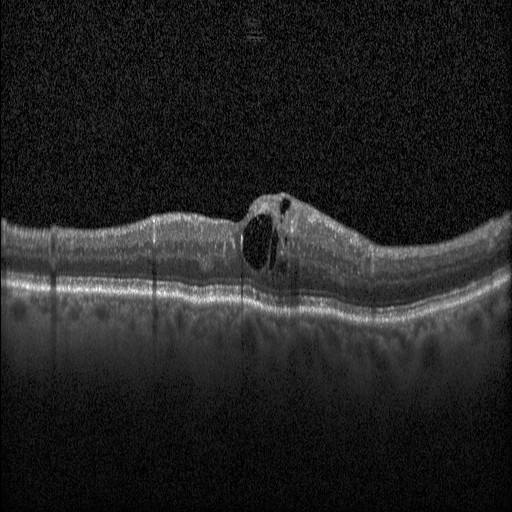
SD-OCT; optical coherence tomography B-scan; through the macula; Heidelberg Spectralis OCT system — Finding: diabetic macular edema.